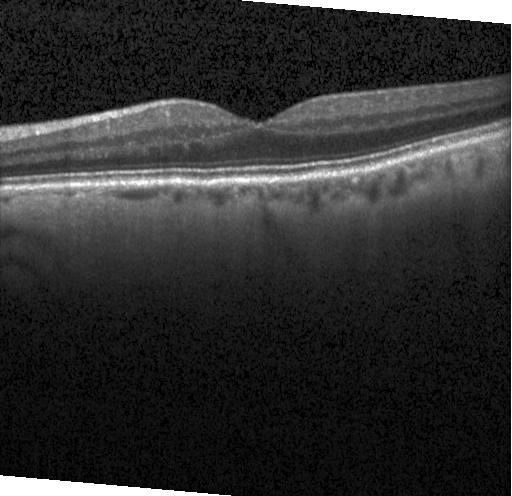

Optical coherence tomography B-scan — Impression: no choroidal neovascularization, diabetic macular edema, or drusen.